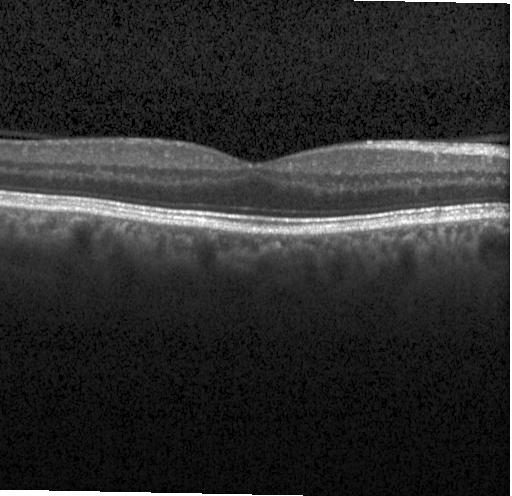 OCT finding: no evidence of choroidal neovascularization, diabetic macular edema, or drusen.